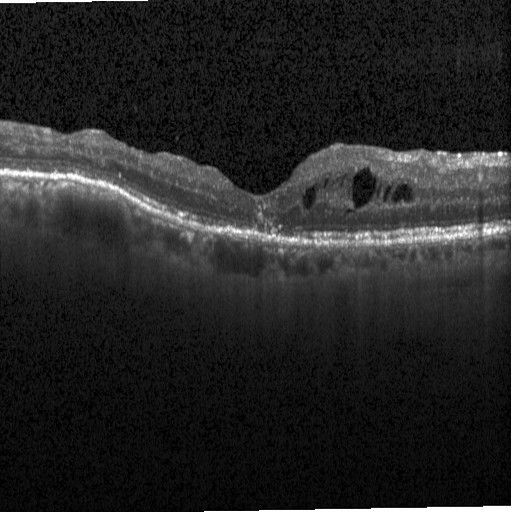
Macular scan. Retinal OCT cross-section — This B-scan demonstrates DME.